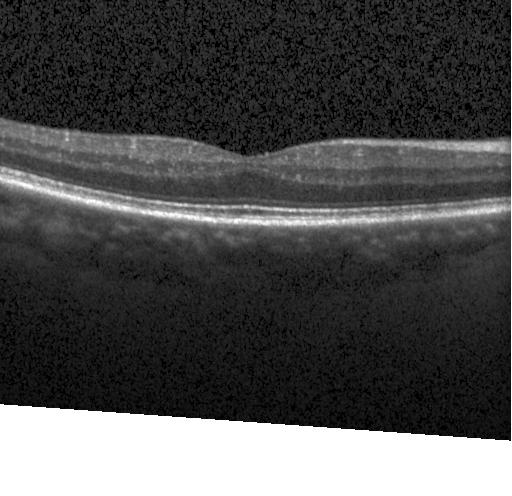 Spectral-domain OCT · OCT line scan — Finding: no evidence of CNV, DME, or drusen.